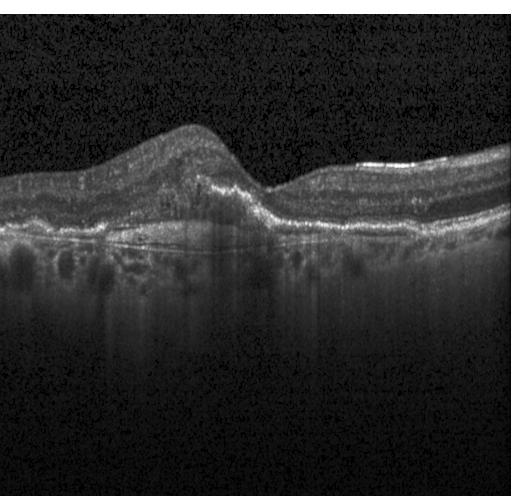

SD-OCT, instrument: Heidelberg Spectralis, OCT B-scan, centered on the fovea
Diagnosis: CNV.